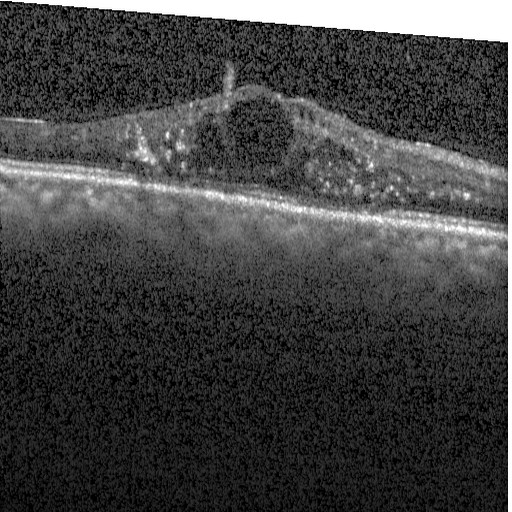
Acquired on a Heidelberg Spectralis. Optical coherence tomography scan. Centered on the fovea. Spectral-domain OCT — Assessment: diabetic macular edema.